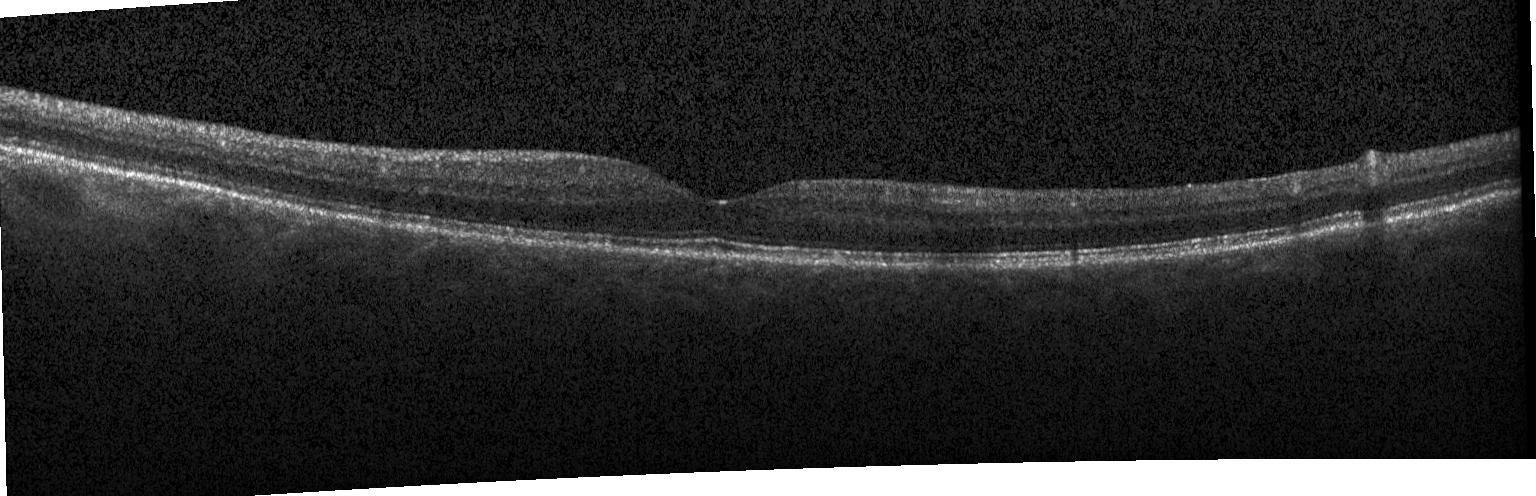

Optical coherence tomography scan · centered on the fovea.
Assessment: no choroidal neovascularization, diabetic macular edema, or drusen.